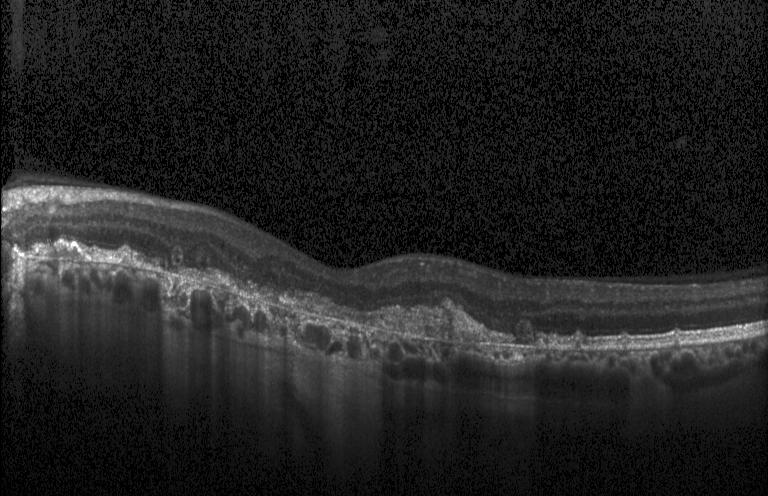

Retinal OCT cross-section
This B-scan demonstrates a choroidal neovascular membrane.